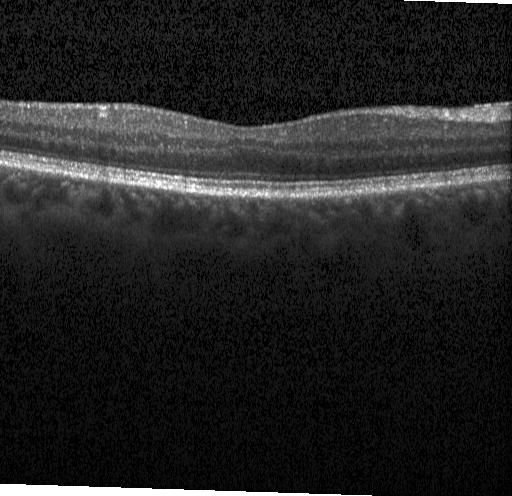
Retinal OCT cross-section; centered on the fovea
Impression: no evidence of choroidal neovascularization, diabetic macular edema, or drusen.